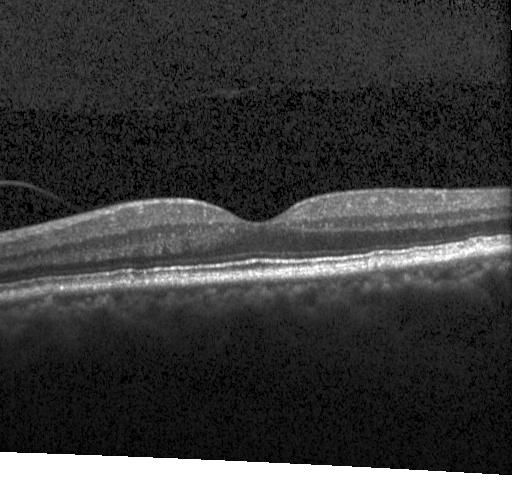
OCT B-scan, through the macula, Heidelberg Spectralis
Assessment: neither choroidal neovascularization, diabetic macular edema, nor drusen.